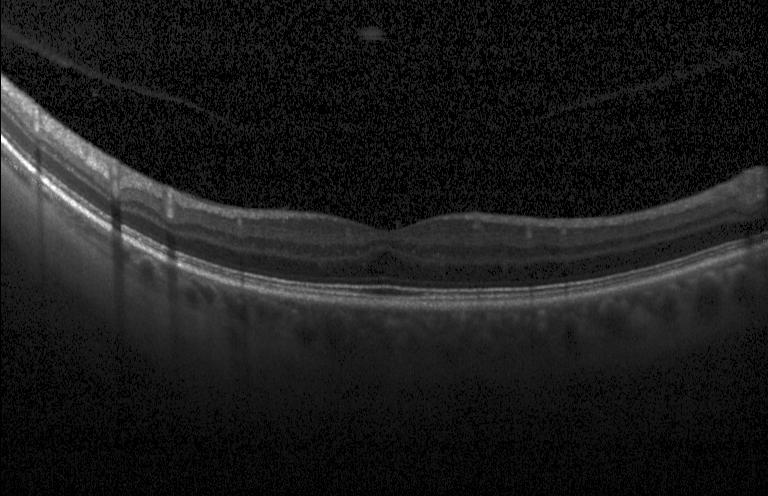
Spectral-domain optical coherence tomography. Heidelberg Spectralis OCT system. Horizontal scan through the fovea. OCT line scan. Diagnosis: no CNV, no DME, and no drusen.